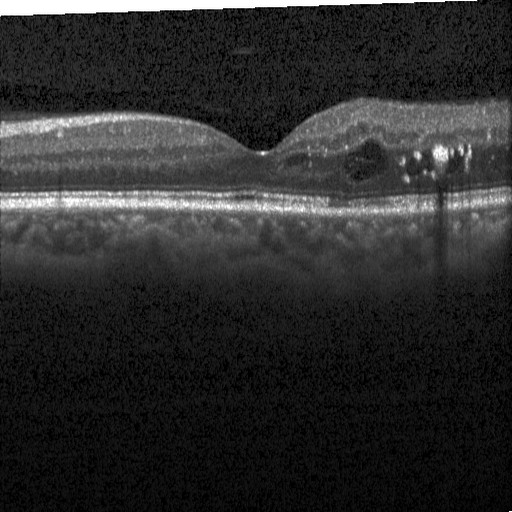 Optical coherence tomography scan — This B-scan demonstrates diabetic macular edema (DME).